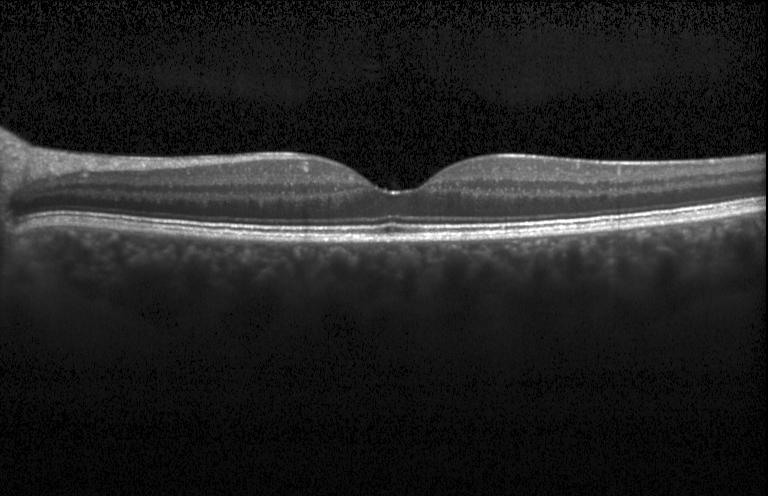 Horizontal scan through the fovea, OCT line scan. Assessment: no evidence of choroidal neovascularization, diabetic macular edema, or drusen.